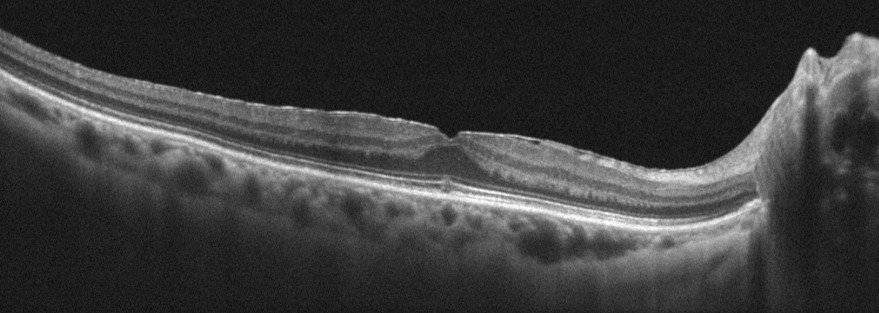 Finding: ERM.